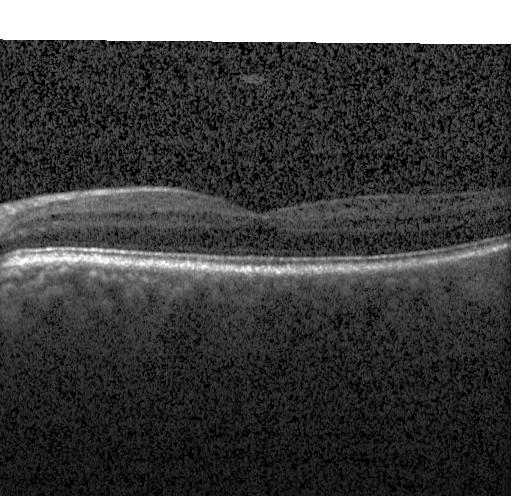
Optical coherence tomography B-scan, SD-OCT, Heidelberg Spectralis
Impression: neither choroidal neovascularization, diabetic macular edema, nor drusen.